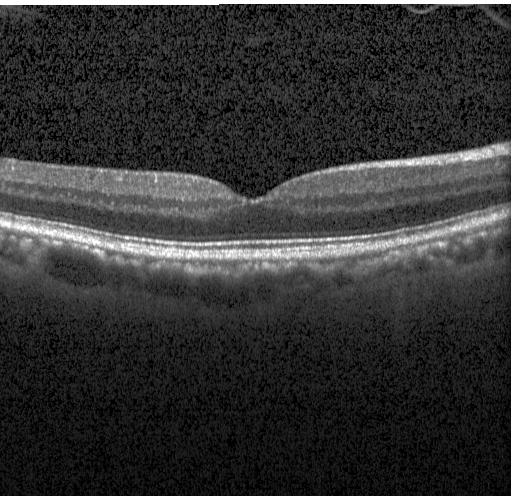 OCT line scan; fovea-centered. Finding: neither choroidal neovascularization, diabetic macular edema, nor drusen.